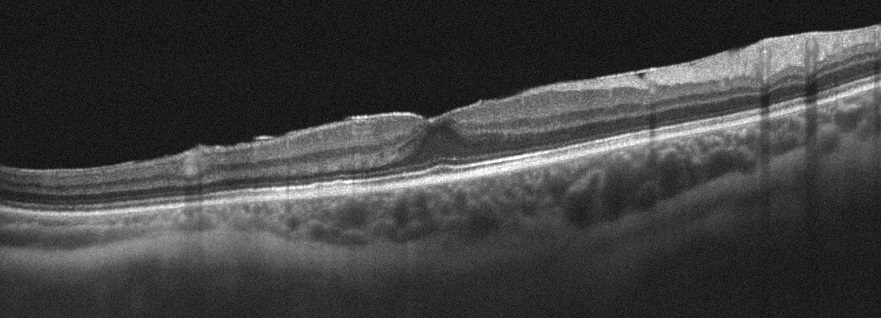

OCT B-scan; instrument: Optovue Avanti RTVue XR. The scan shows ERM.